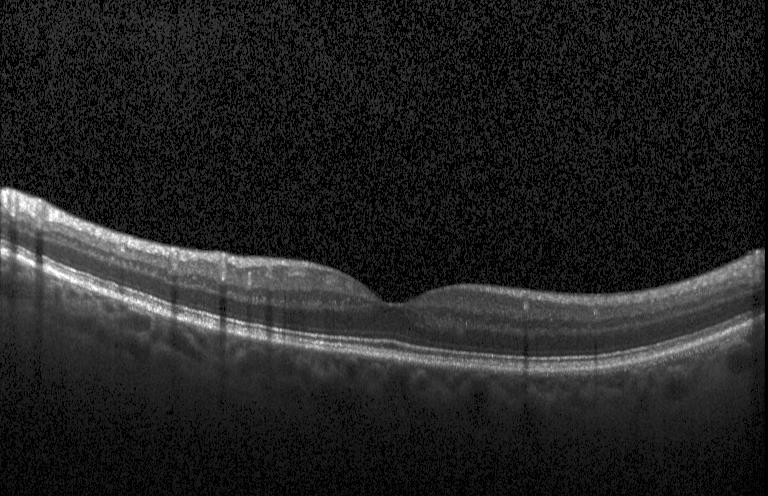
Dx: no choroidal neovascularization, diabetic macular edema, or drusen.